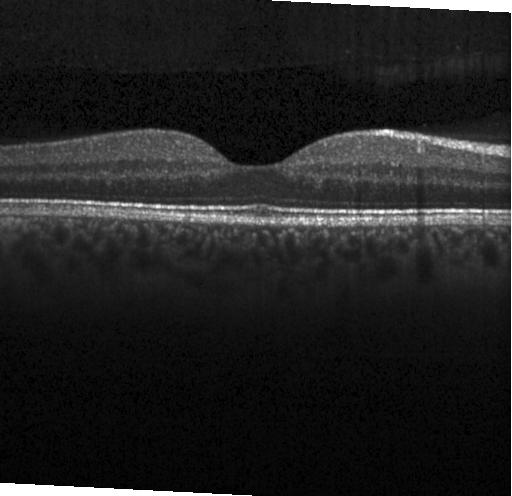
OCT B-scan; spectral-domain optical coherence tomography; Heidelberg Spectralis OCT system; fovea-centered — The scan shows neither choroidal neovascularization, diabetic macular edema, nor drusen.